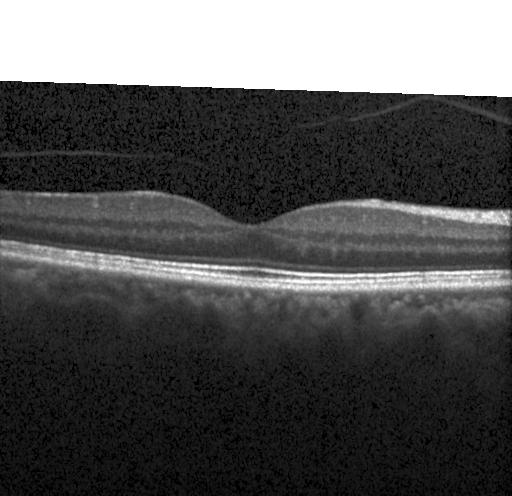

Optical coherence tomography B-scan
Impression: neither CNV, DME, nor drusen.